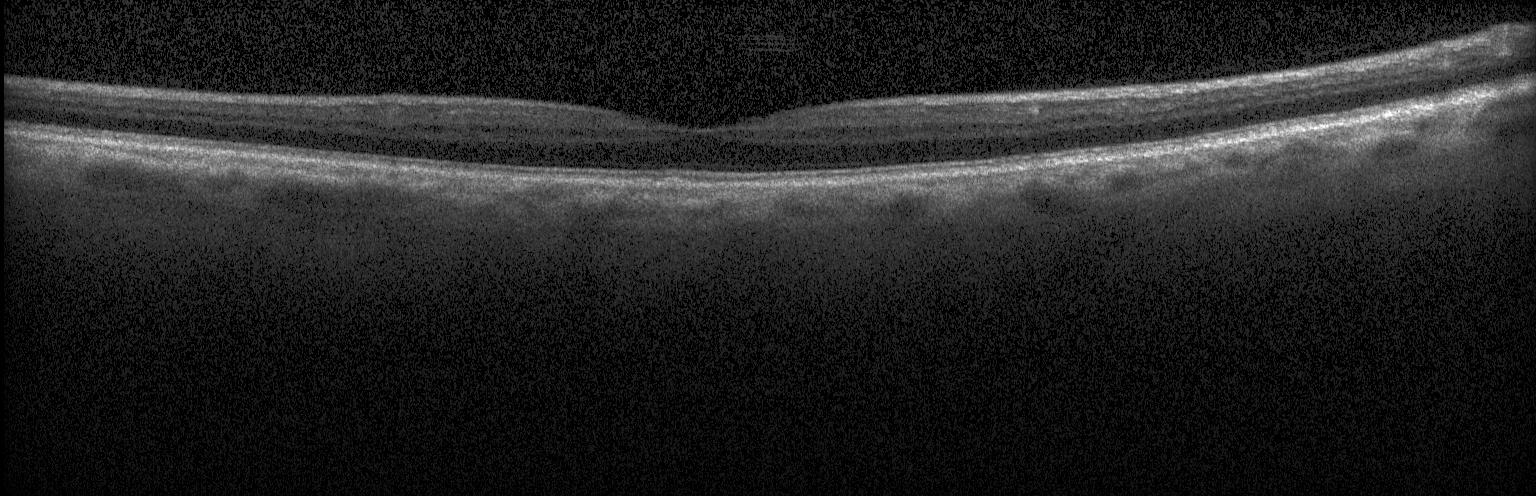
Instrument: Heidelberg Spectralis. Through the macula. Optical coherence tomography B-scan
Macular OCT: no CNV, DME, or drusen.